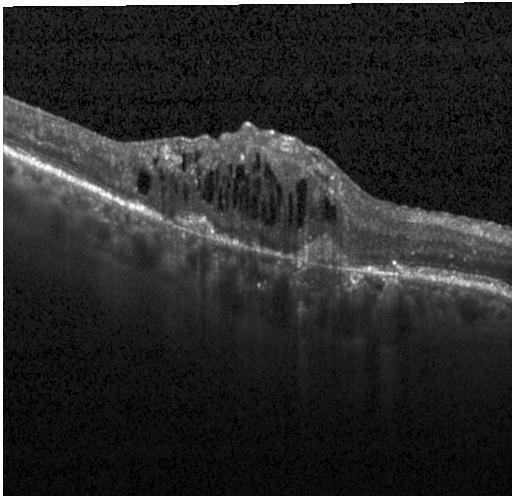

OCT finding: CNV.